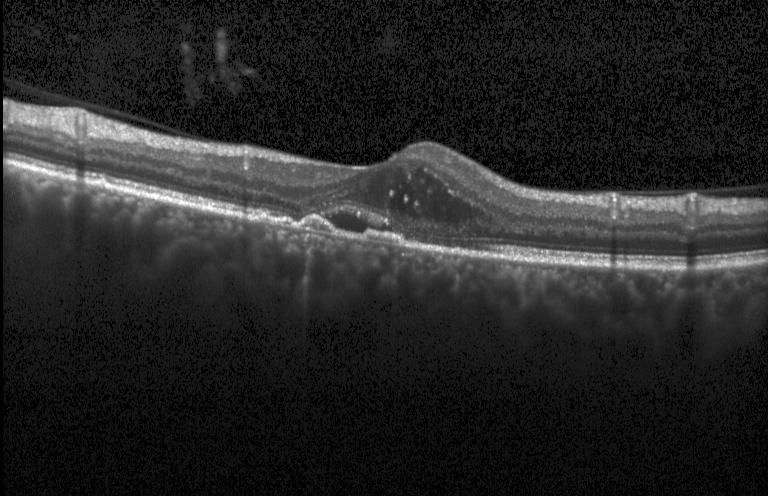
OCT finding: CNV.